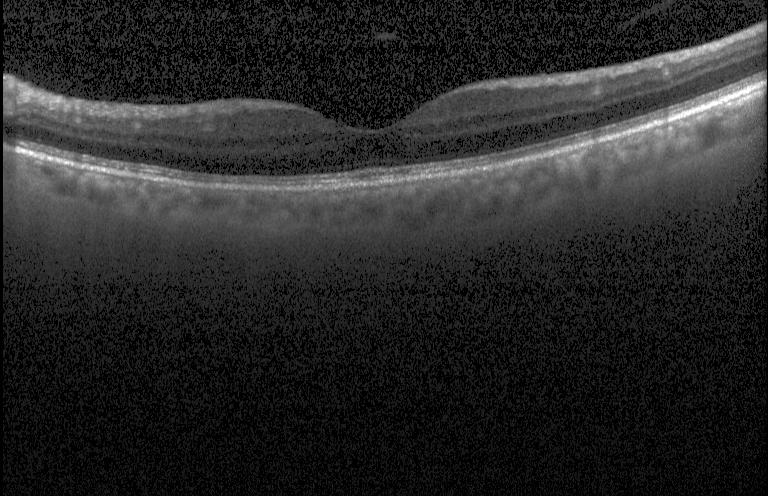
OCT finding: neither choroidal neovascularization, diabetic macular edema, nor drusen.